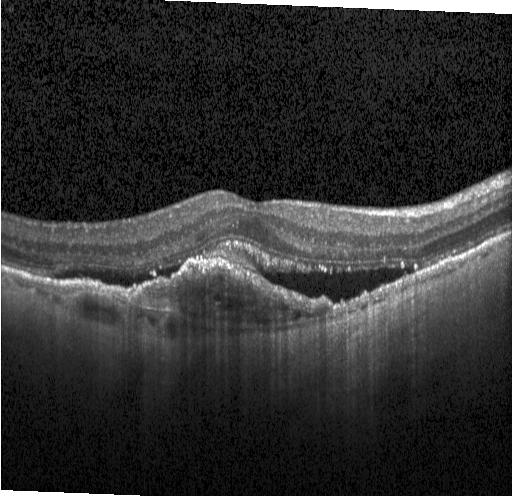 Assessment: a choroidal neovascular membrane.